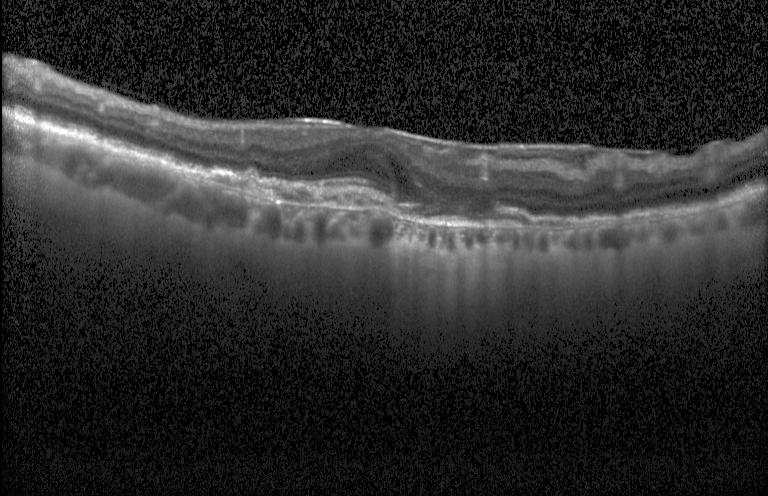

Macular OCT demonstrating a choroidal neovascular membrane.